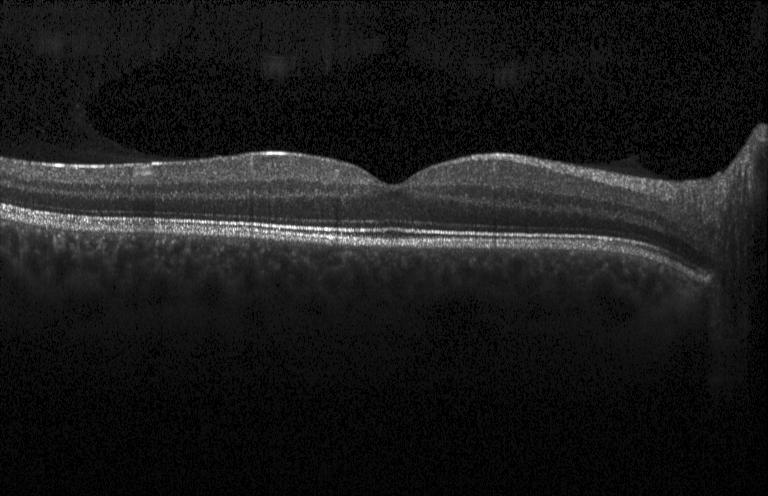 OCT finding: no CNV, no DME, and no drusen.